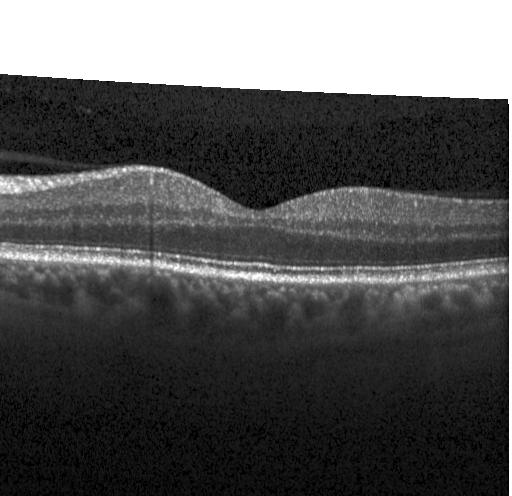

Macular OCT: neither choroidal neovascularization, diabetic macular edema, nor drusen.